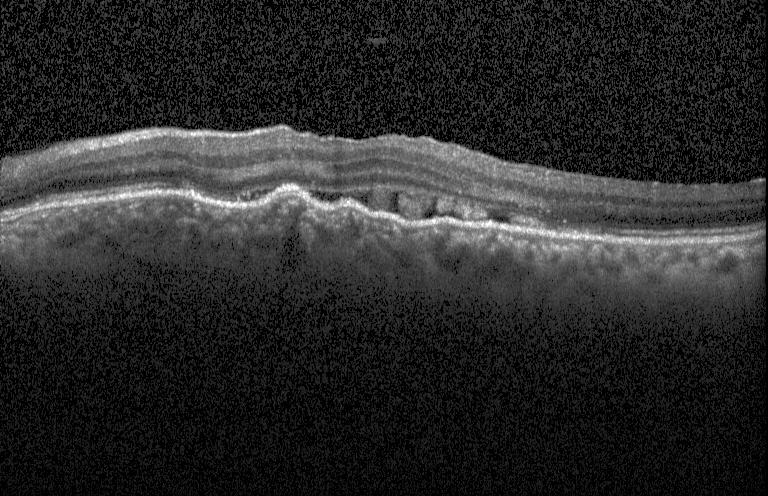 Diagnosis: a choroidal neovascular membrane.